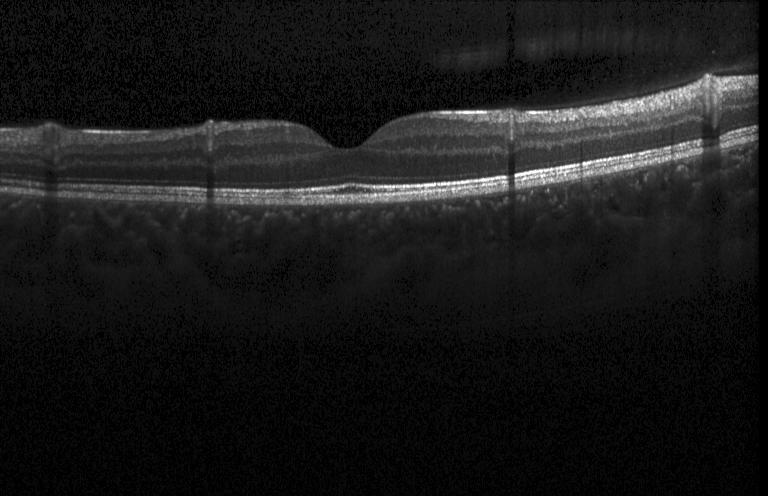
Retinal OCT B-scan · horizontal scan through the fovea.
Impression: neither CNV, DME, nor drusen.